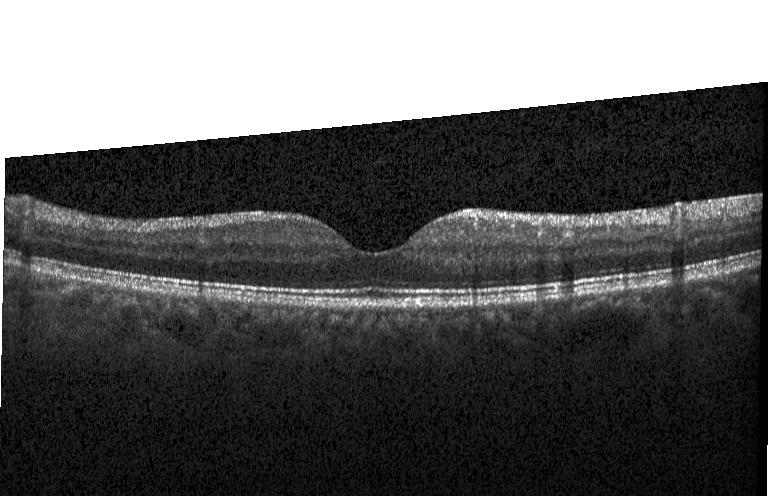 Spectral-domain OCT; retinal OCT cross-section; instrument: Heidelberg Spectralis; macular scan.
This B-scan demonstrates no choroidal neovascularization, diabetic macular edema, or drusen.